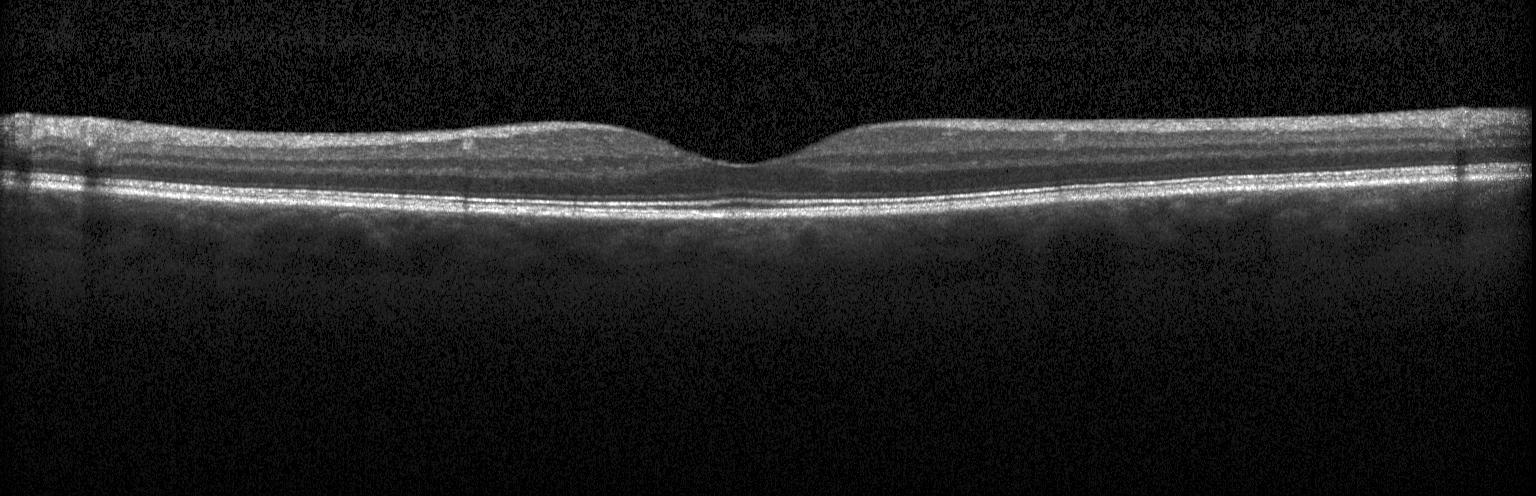

OCT line scan.
Dx: no CNV, no DME, and no drusen.